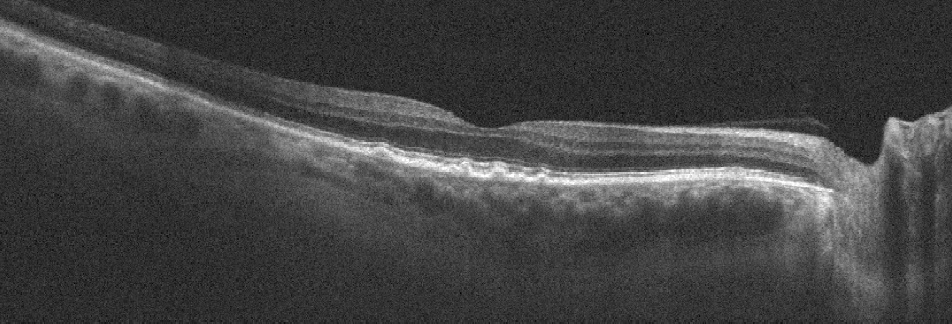
Diagnosis: age-related macular degeneration.